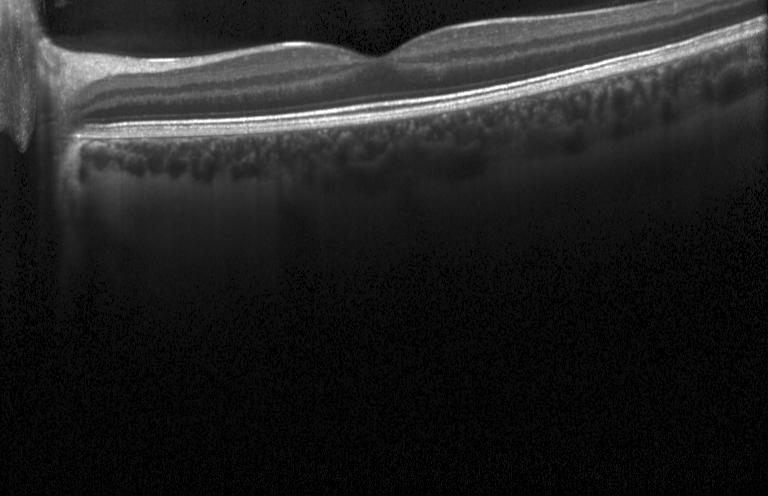
Finding: no evidence of CNV, DME, or drusen.